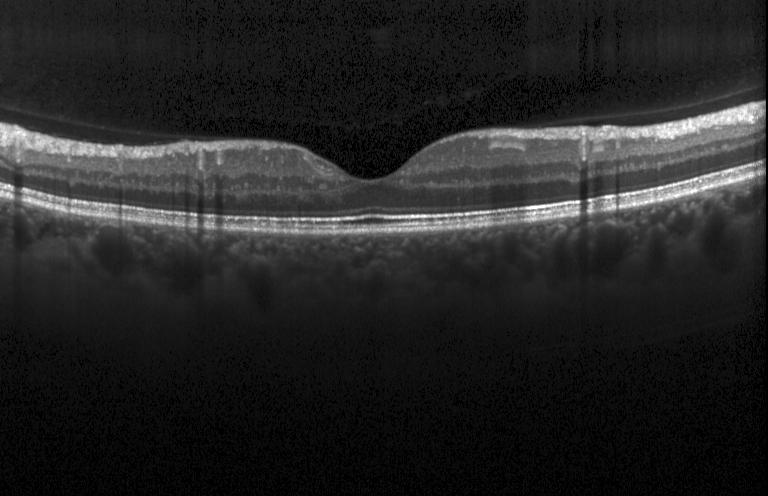

Assessment: no CNV, no DME, and no drusen.